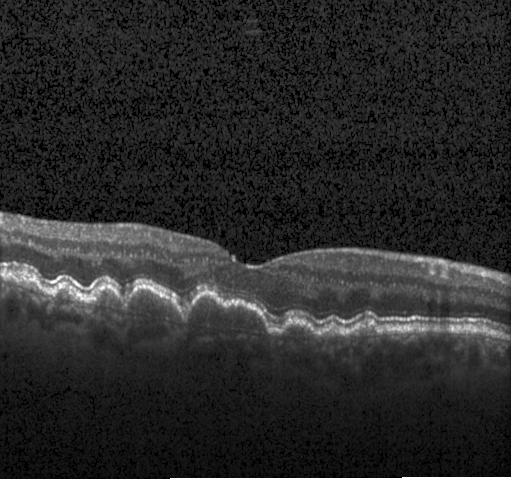 Centered on the fovea, SD-OCT, OCT line scan, Heidelberg Spectralis OCT system.
The scan shows drusen.